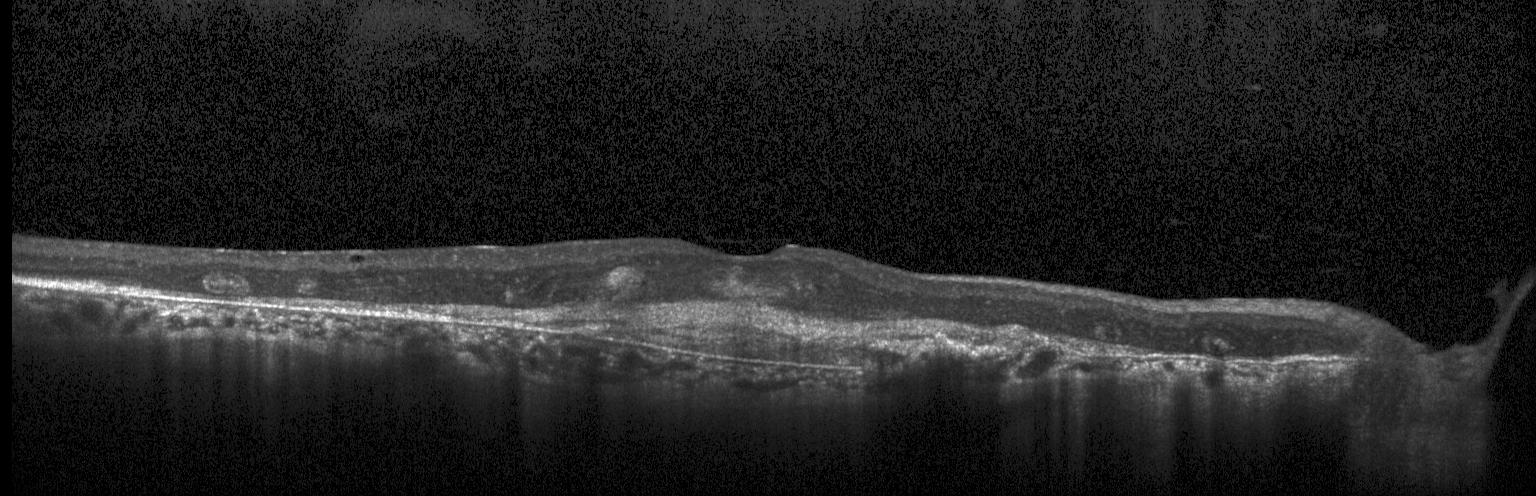

OCT B-scan showing CNV.